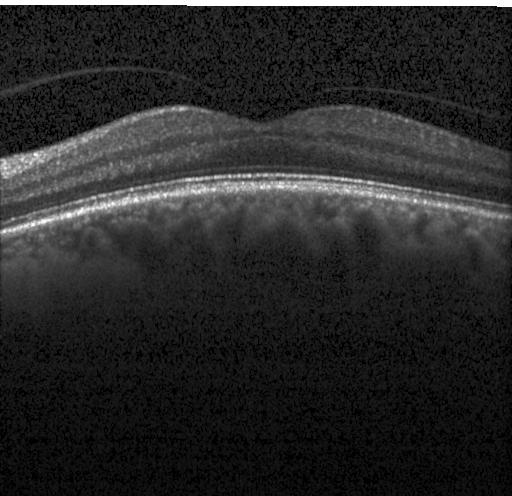

Optical coherence tomography scan
Finding: no CNV, DME, or drusen.